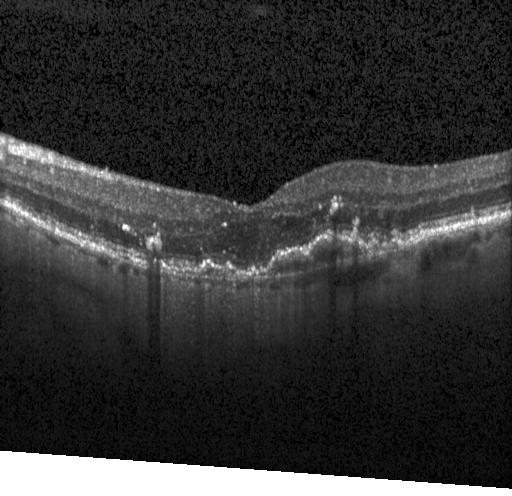
Retinal OCT B-scan
Finding: choroidal neovascularization.